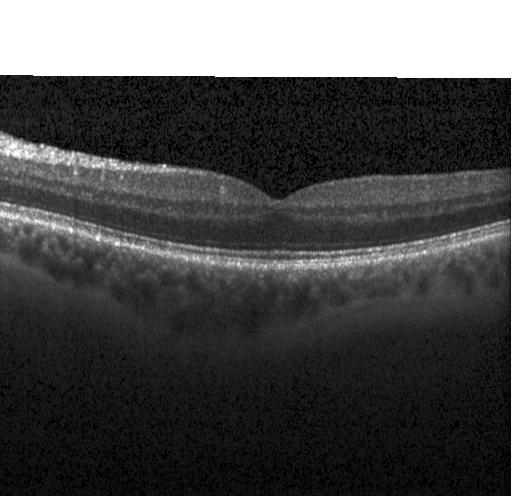 Spectral-domain optical coherence tomography; macular scan; optical coherence tomography B-scan.
OCT finding: no choroidal neovascularization, no diabetic macular edema, and no drusen.